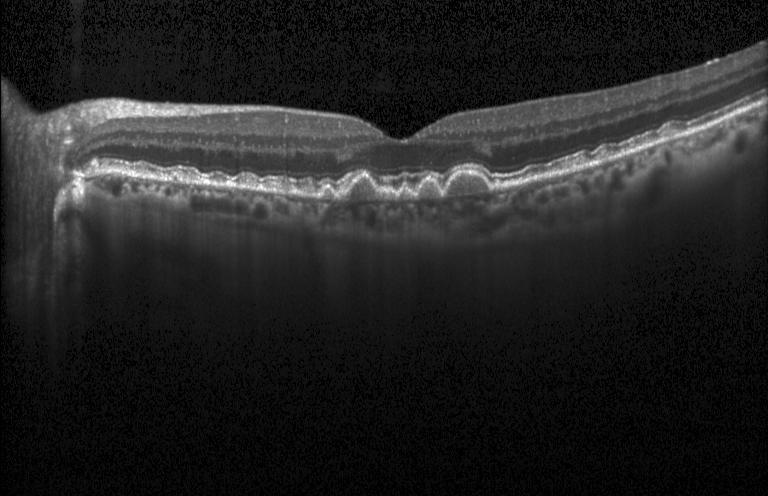 Macular OCT: sub-RPE drusenoid deposits.